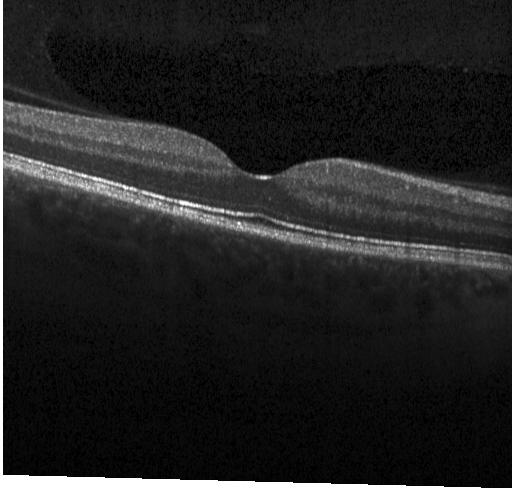 Assessment: no choroidal neovascularization, no diabetic macular edema, and no drusen.